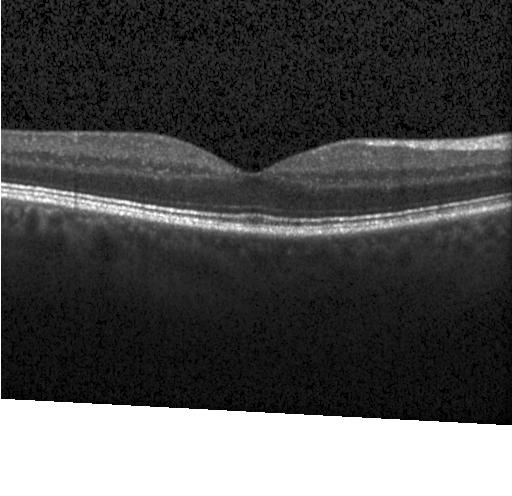
Optical coherence tomography scan, spectral-domain OCT
The scan shows no choroidal neovascularization, diabetic macular edema, or drusen.